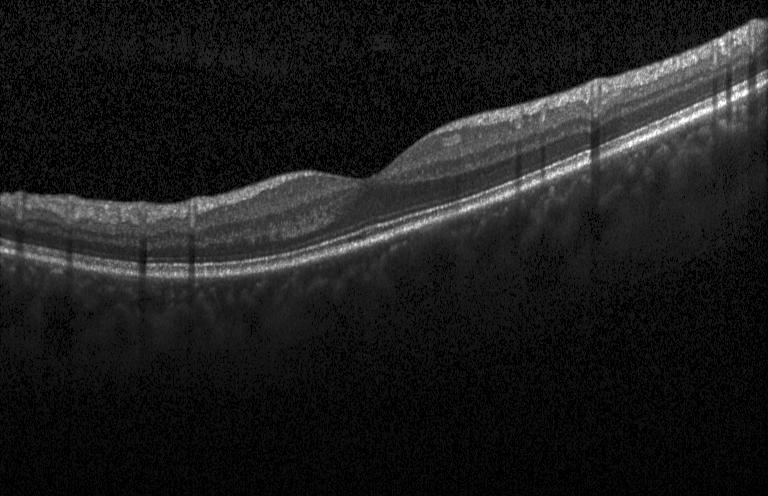
Diagnosis: neither choroidal neovascularization, diabetic macular edema, nor drusen.